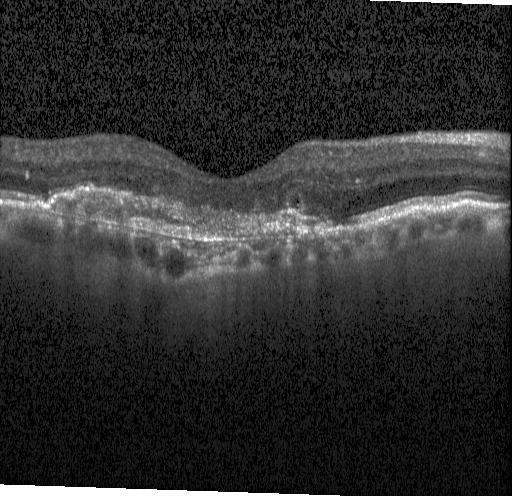

Retinal OCT cross-section; horizontal scan through the fovea; spectral-domain OCT.
Macular OCT: choroidal neovascularization (CNV).